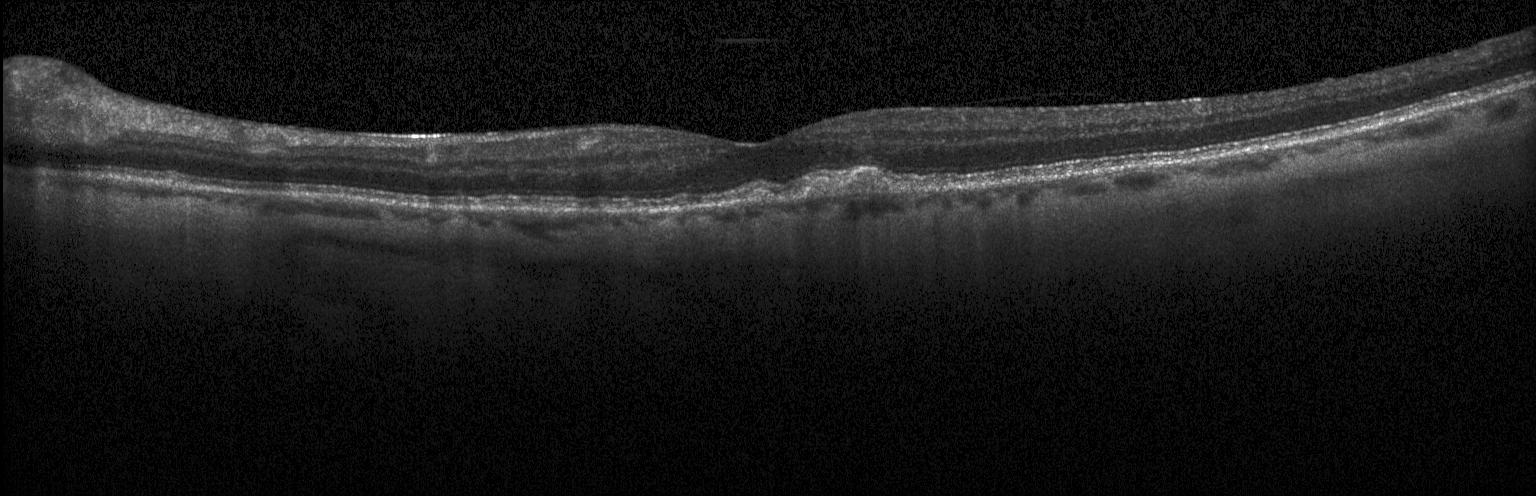 Through the macula, OCT line scan, spectral-domain OCT.
Dx: a choroidal neovascular membrane.